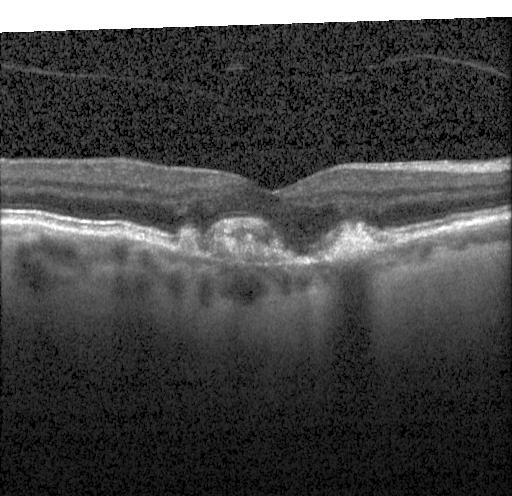
Dx: a choroidal neovascular membrane.